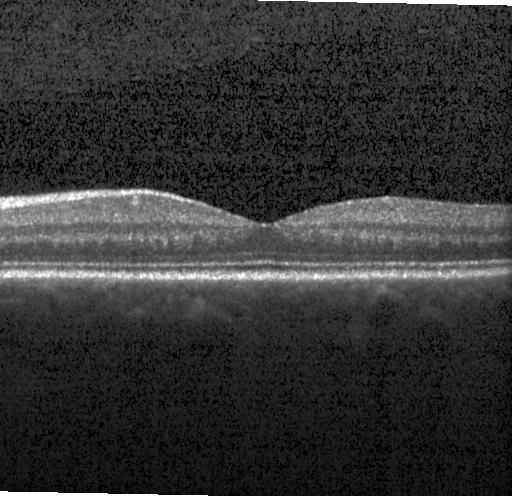 Optical coherence tomography scan; spectral-domain optical coherence tomography; acquired on a Heidelberg Spectralis
Finding: no choroidal neovascularization, diabetic macular edema, or drusen.